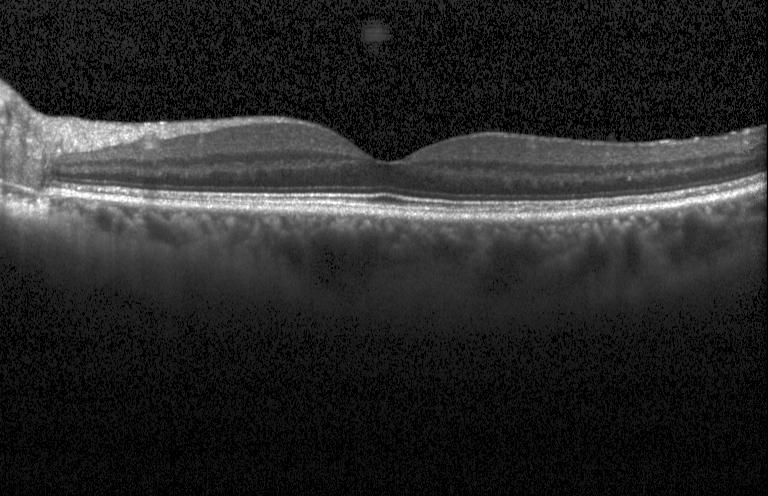
Retinal OCT B-scan.
Finding: no evidence of choroidal neovascularization, diabetic macular edema, or drusen.